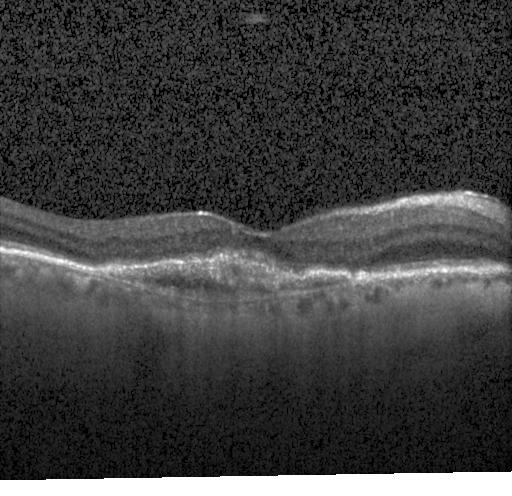
Spectral-domain OCT · OCT B-scan.
This B-scan demonstrates a choroidal neovascular membrane.